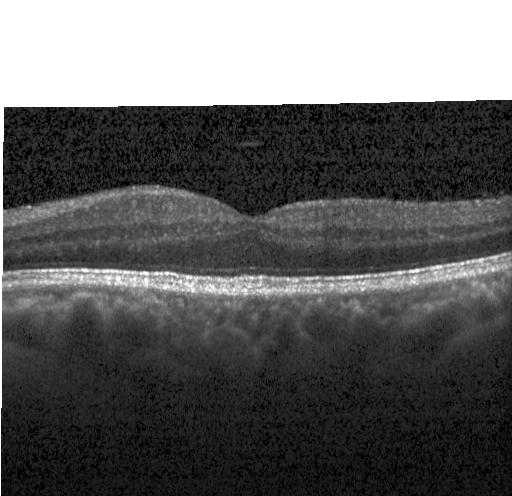
Dx: no choroidal neovascularization, diabetic macular edema, or drusen.